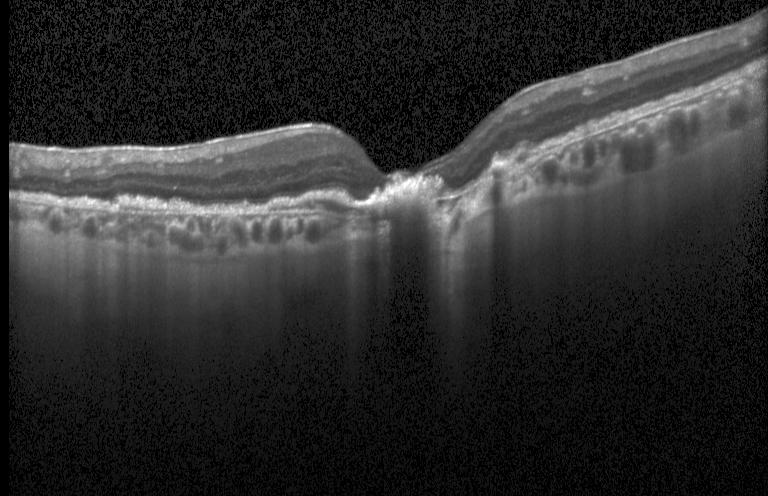
SD-OCT, optical coherence tomography scan, centered on the fovea, acquired on a Heidelberg Spectralis.
Choroidal neovascularization (CNV).